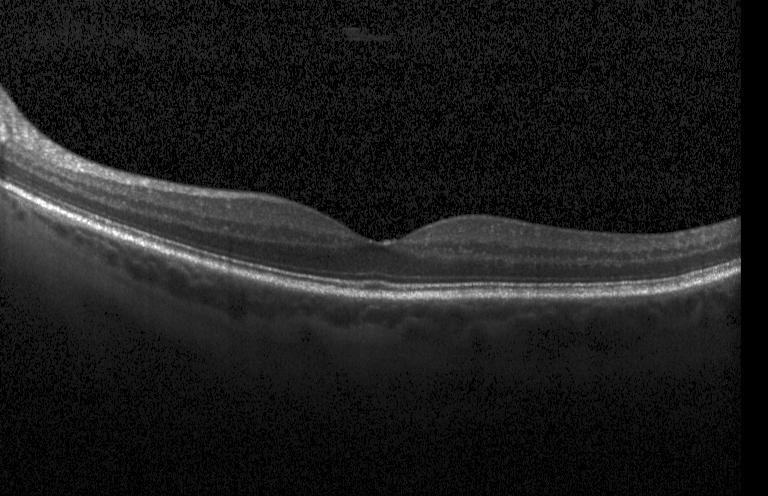 OCT B-scan
Diagnosis: no evidence of choroidal neovascularization, diabetic macular edema, or drusen.